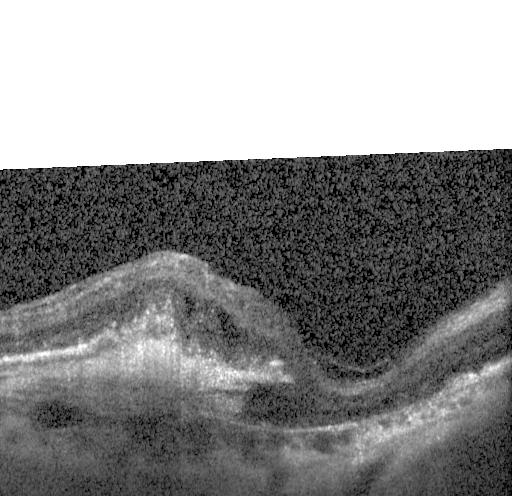

Impression: choroidal neovascularization.